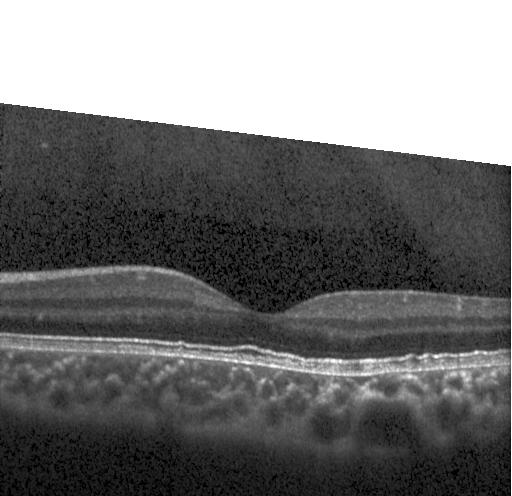
Finding: neither choroidal neovascularization, diabetic macular edema, nor drusen.